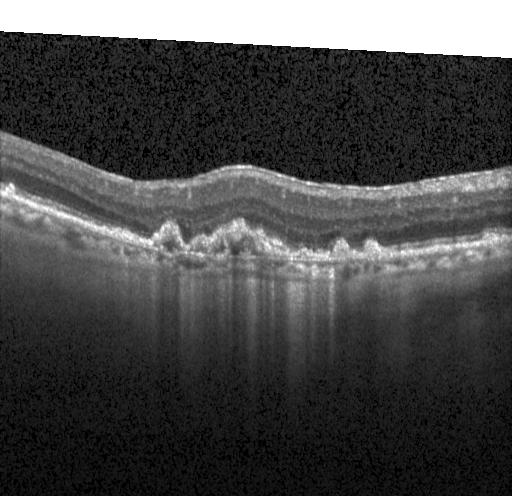 OCT B-scan; spectral-domain OCT; Heidelberg Spectralis OCT system; macular scan — The scan shows CNV.